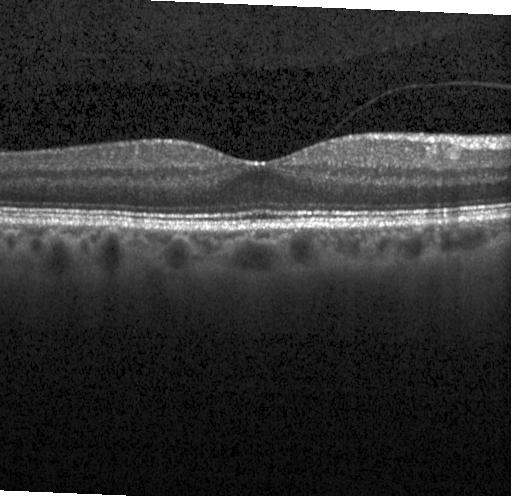
Instrument: Heidelberg Spectralis; retinal OCT B-scan; spectral-domain optical coherence tomography. Neither choroidal neovascularization, diabetic macular edema, nor drusen.